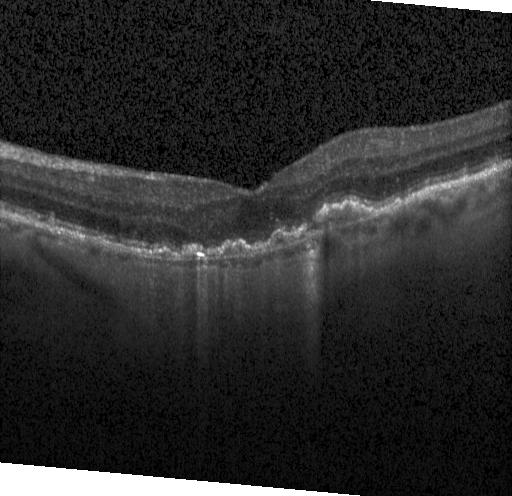 Diagnosis: CNV.